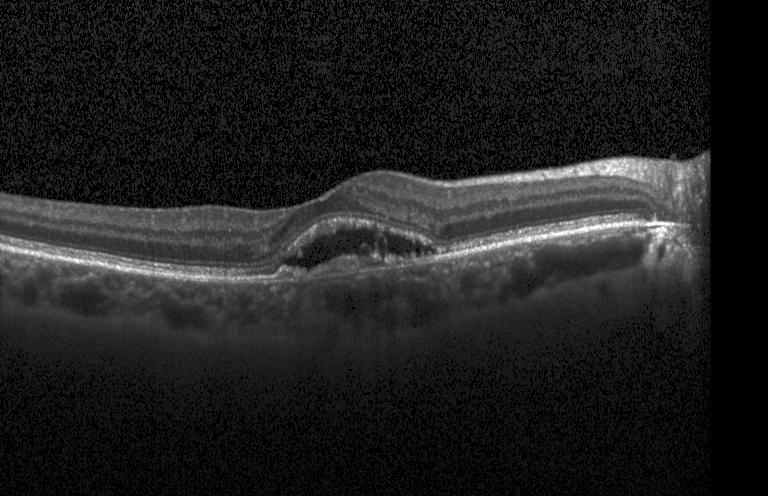

Finding: choroidal neovascularization.